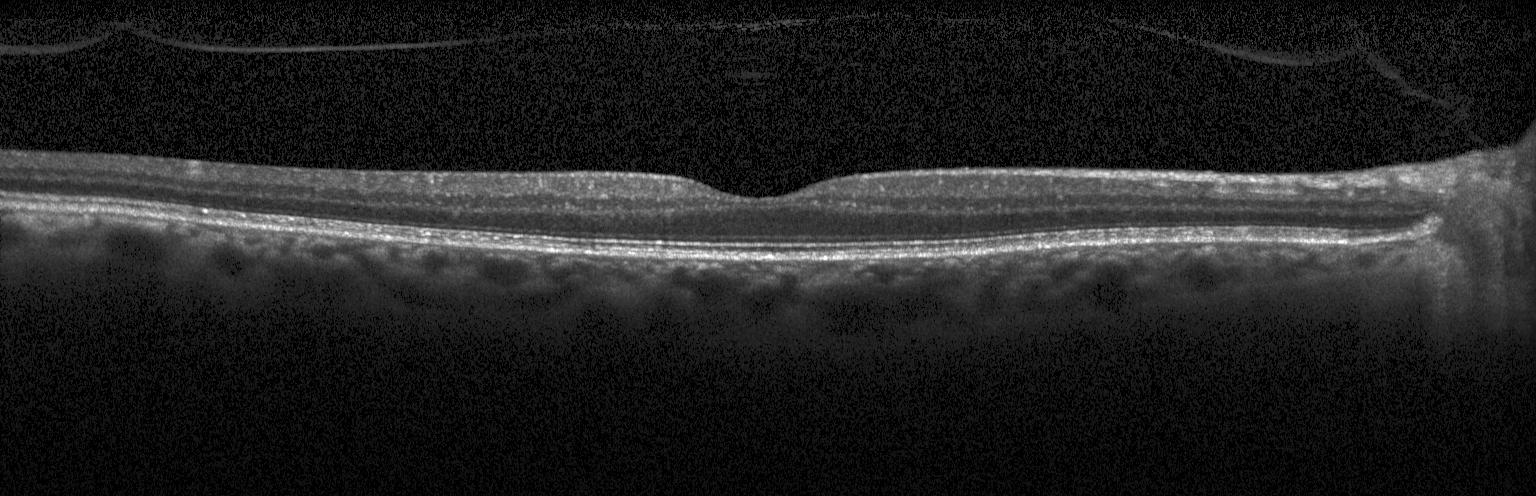
Retinal OCT cross-section; spectral-domain OCT; Heidelberg Spectralis.
Macular OCT: no choroidal neovascularization, diabetic macular edema, or drusen.